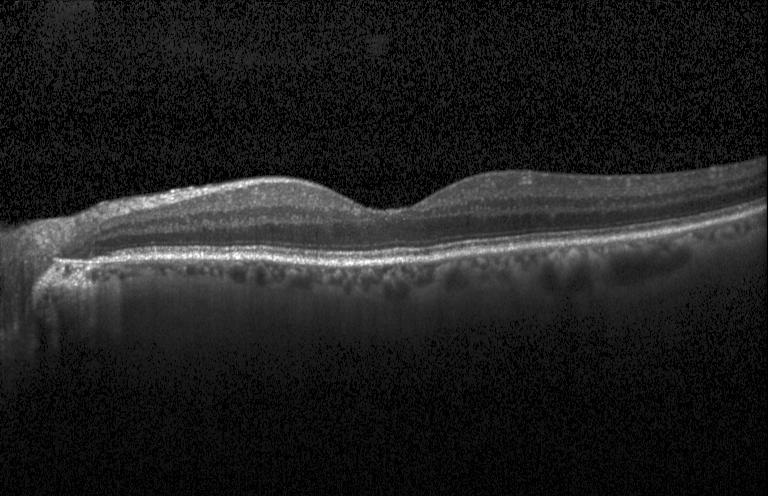 Macular scan; OCT line scan; SD-OCT; acquired on a Heidelberg Spectralis. OCT finding: no choroidal neovascularization, diabetic macular edema, or drusen.